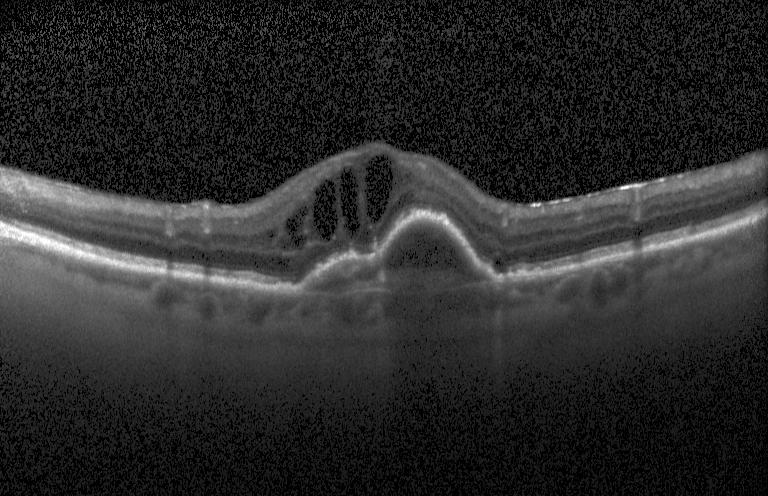 OCT scan showing a choroidal neovascular membrane.